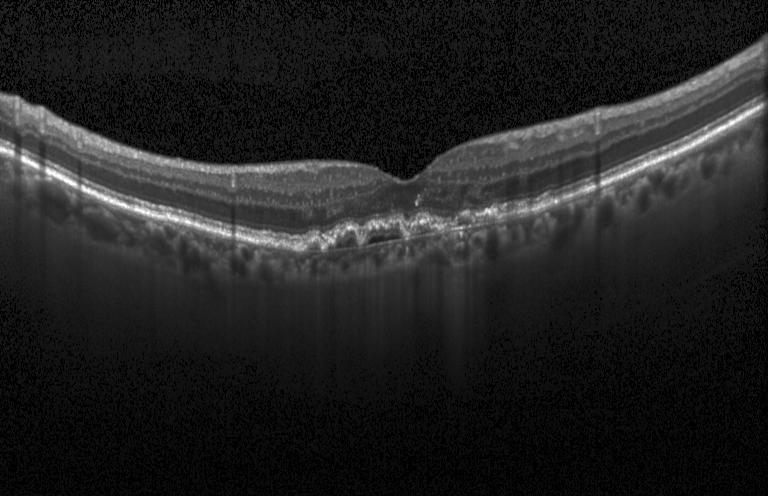 Retinal OCT B-scan · spectral-domain optical coherence tomography — Diagnosis: a choroidal neovascular membrane.